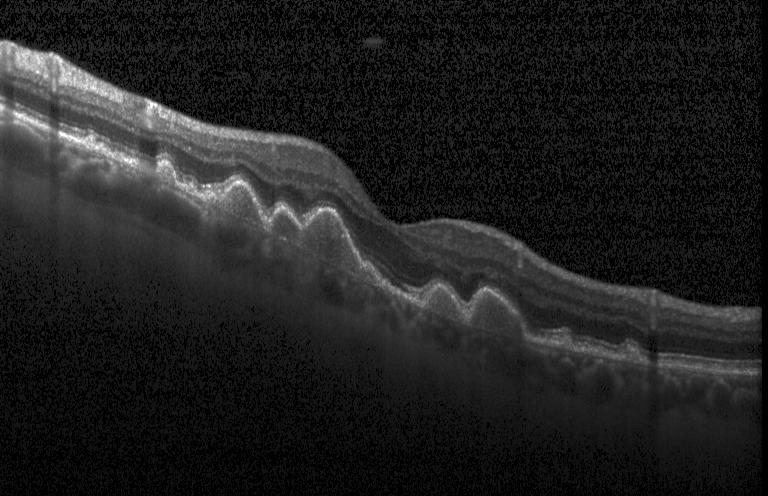

Retinal OCT B-scan, spectral-domain optical coherence tomography, centered on the fovea — Diagnosis: drusen.